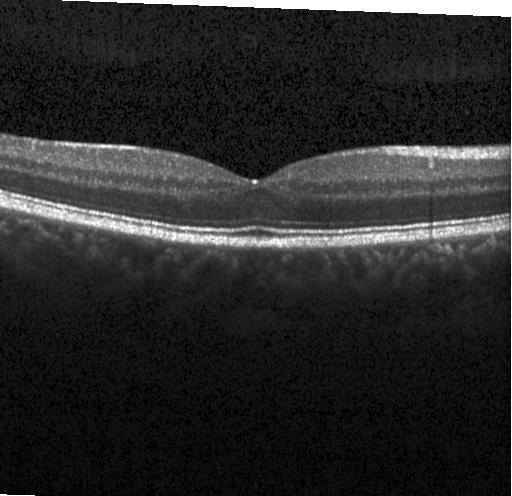 Retinal OCT B-scan. Spectral-domain OCT.
No CNV, no DME, and no drusen.